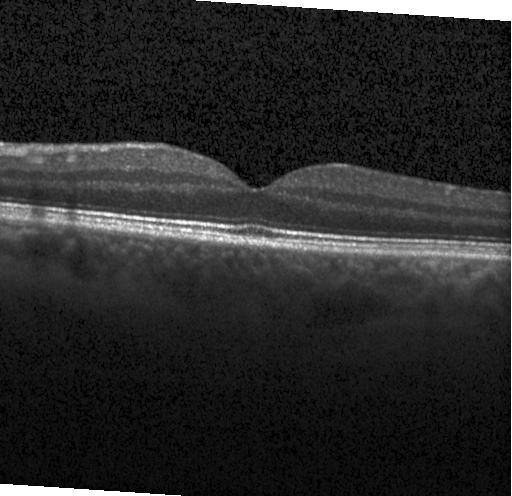
Assessment: no choroidal neovascularization, diabetic macular edema, or drusen.